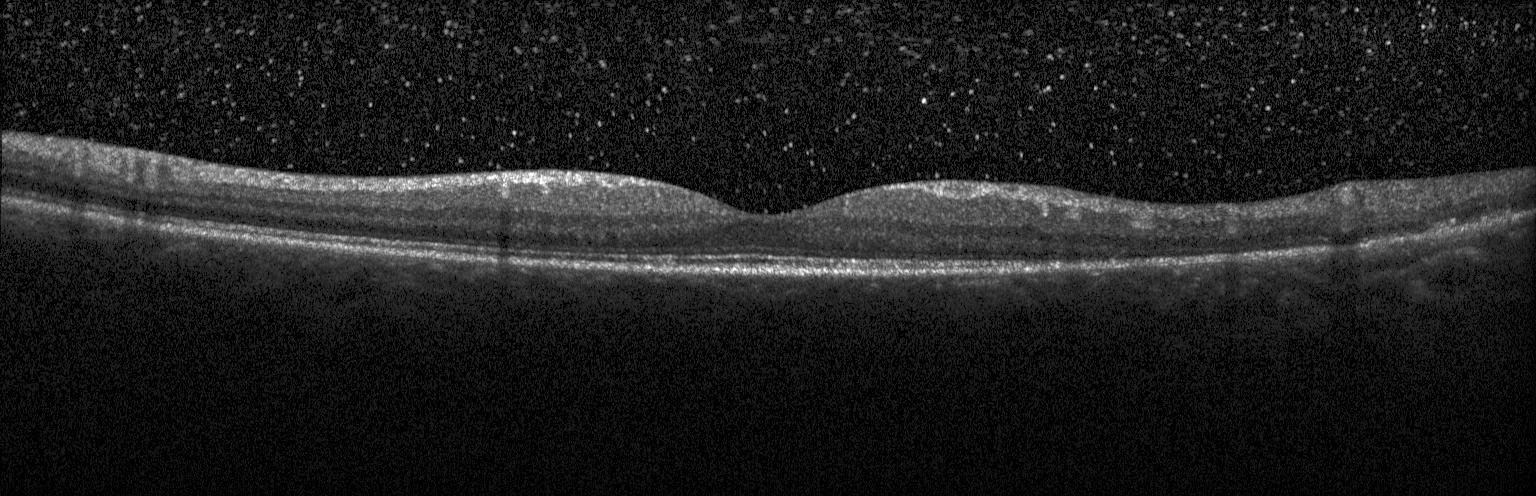

OCT B-scan showing neither CNV, DME, nor drusen.